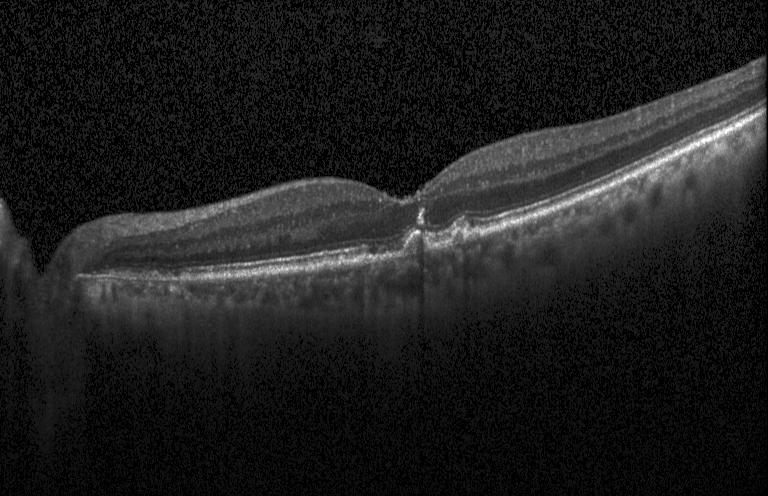
Spectral-domain OCT B-scan: drusen.